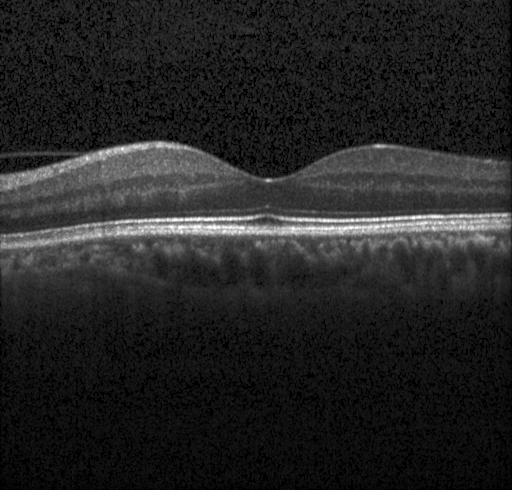
OCT scan showing neither CNV, DME, nor drusen.